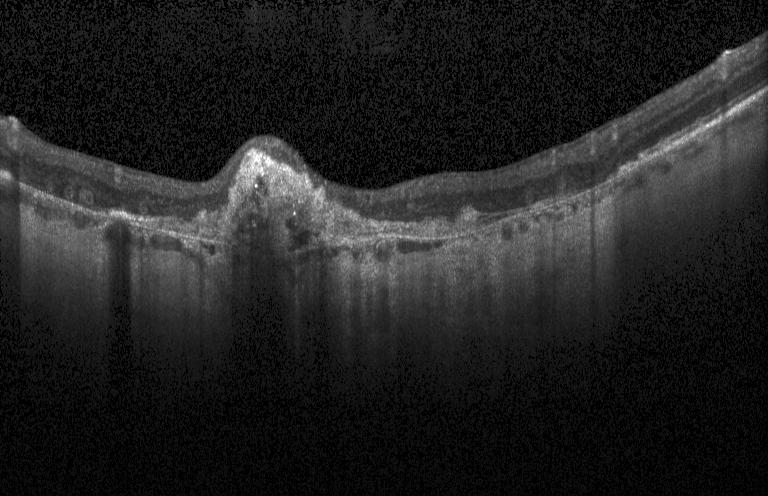
Macular OCT demonstrating CNV.